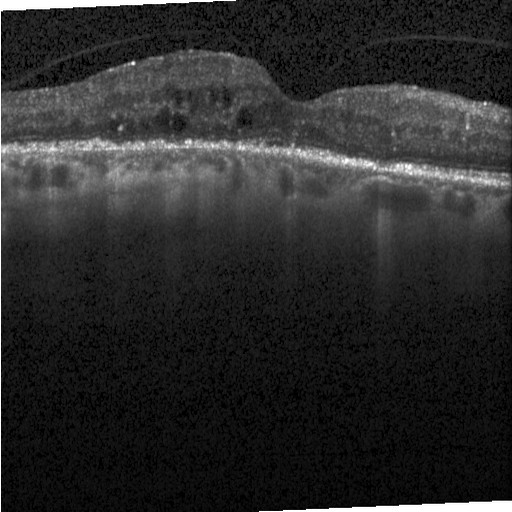

OCT line scan. Assessment: diabetic macular edema (DME).